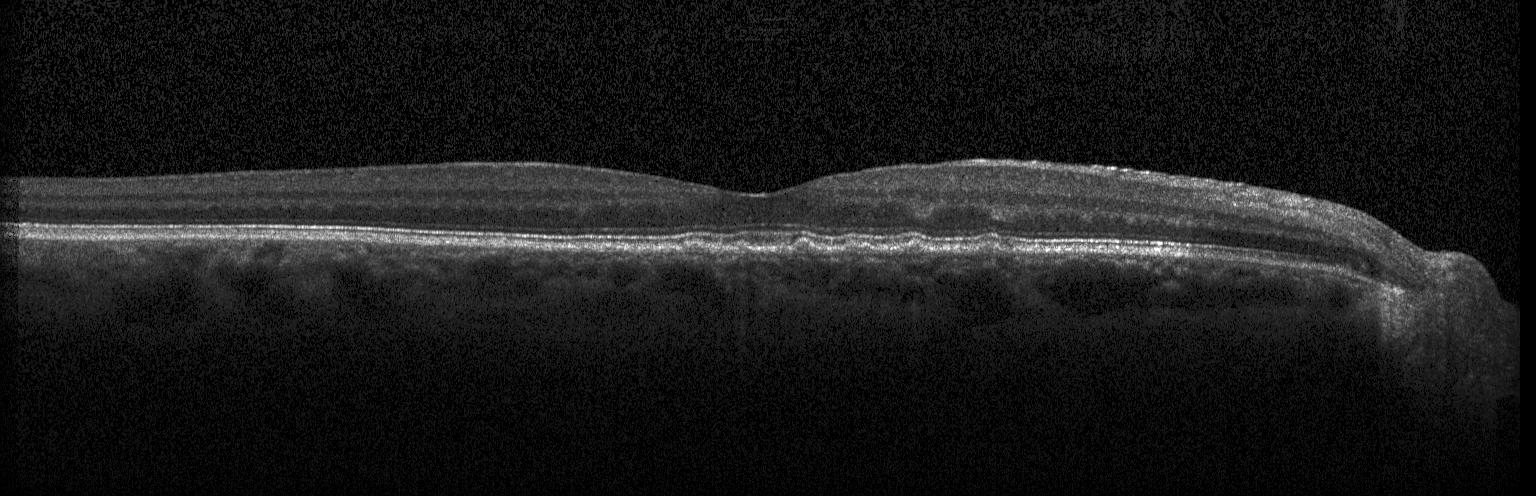 Through the macula · OCT B-scan
Assessment: sub-RPE drusenoid deposits.